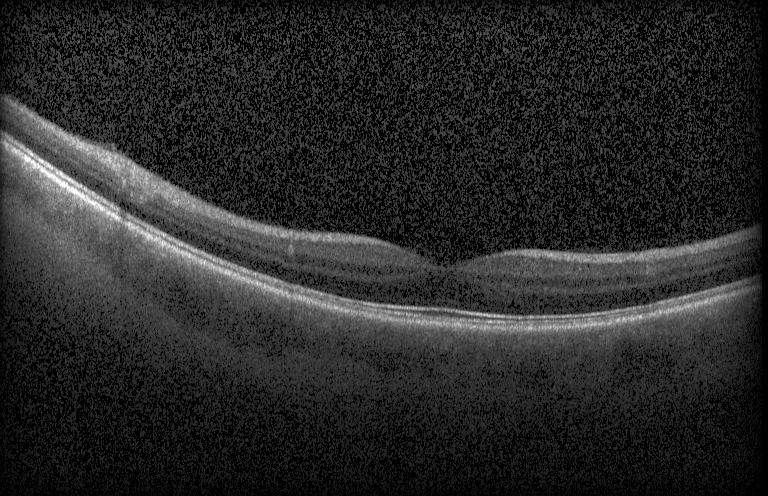

OCT finding: neither choroidal neovascularization, diabetic macular edema, nor drusen.